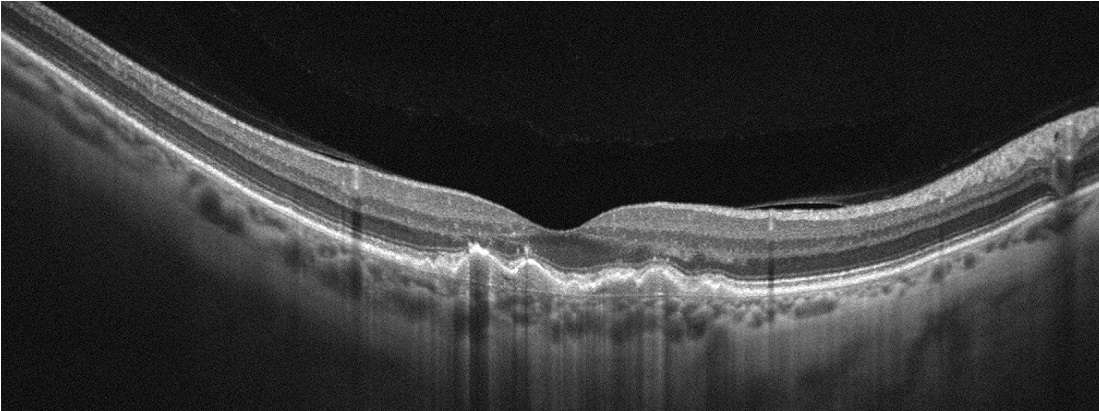

Retinal OCT cross-section showing age-related macular degeneration.